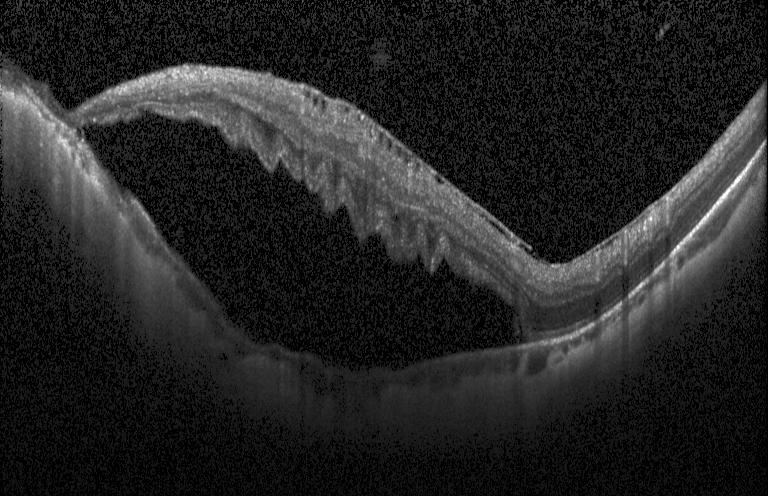 SD-OCT · optical coherence tomography scan.
Impression: choroidal neovascularization.